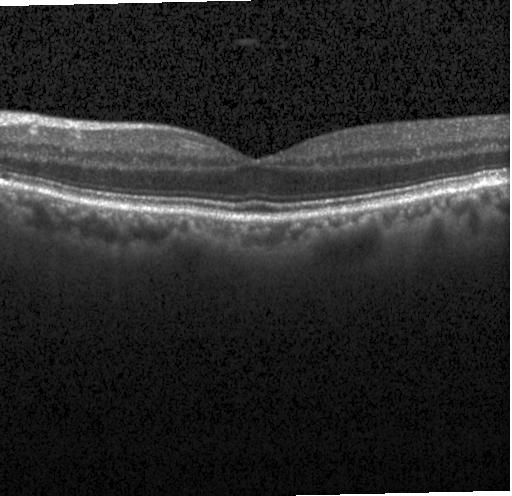 Diagnosis: no CNV, DME, or drusen.